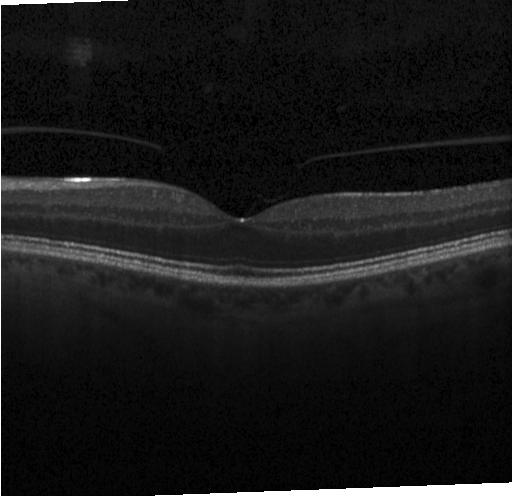 The scan shows no evidence of choroidal neovascularization, diabetic macular edema, or drusen.